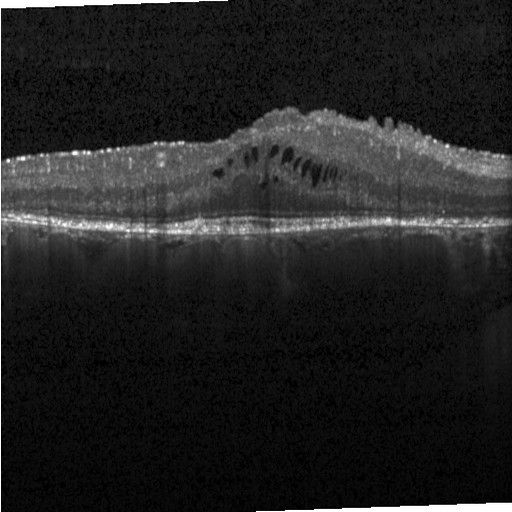 OCT line scan, macular scan, Heidelberg Spectralis OCT system — Finding: diabetic macular edema (DME).